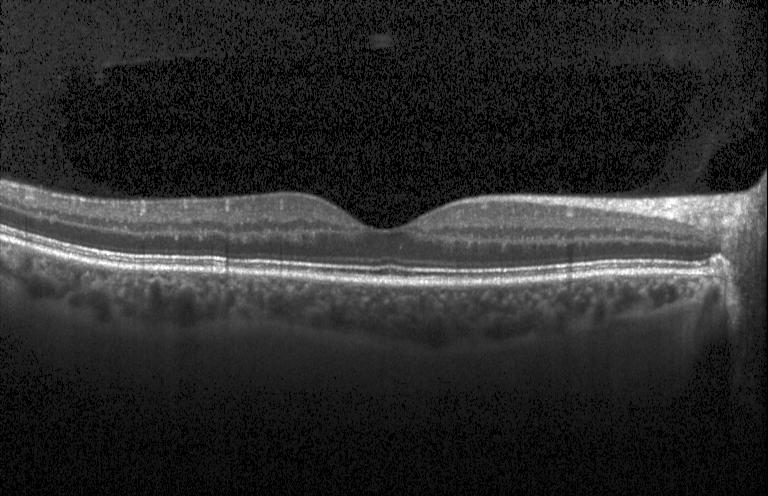 OCT finding: no CNV, DME, or drusen.